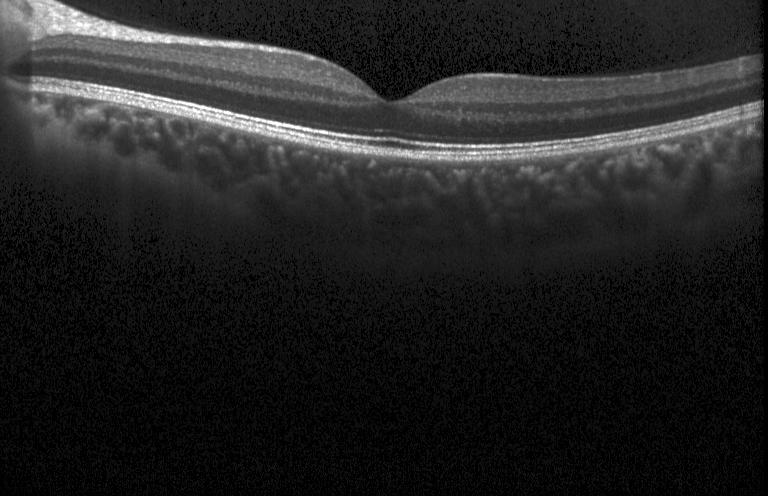

Through the macula, spectral-domain optical coherence tomography, OCT line scan, Heidelberg Spectralis
The scan shows no choroidal neovascularization, no diabetic macular edema, and no drusen.